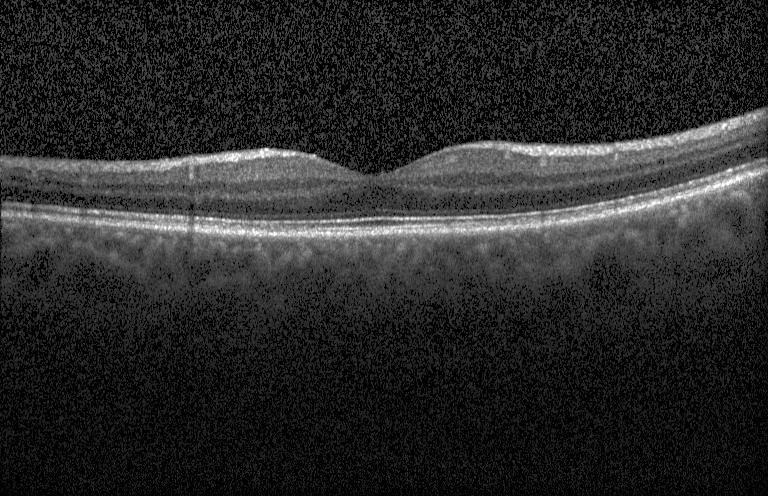

Retinal OCT cross-section, SD-OCT, instrument: Heidelberg Spectralis, fovea-centered.
Assessment: no choroidal neovascularization, diabetic macular edema, or drusen.